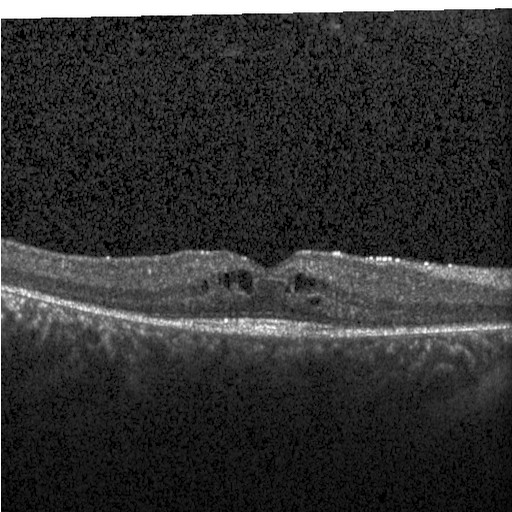
Optical coherence tomography B-scan · fovea-centered · acquired on a Heidelberg Spectralis · SD-OCT. OCT finding: DME.